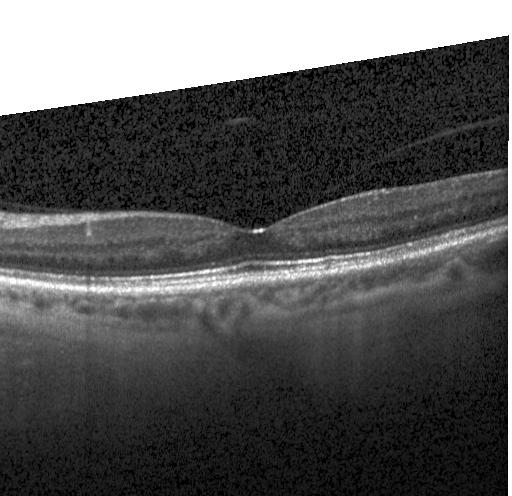
OCT scan showing no CNV, DME, or drusen.